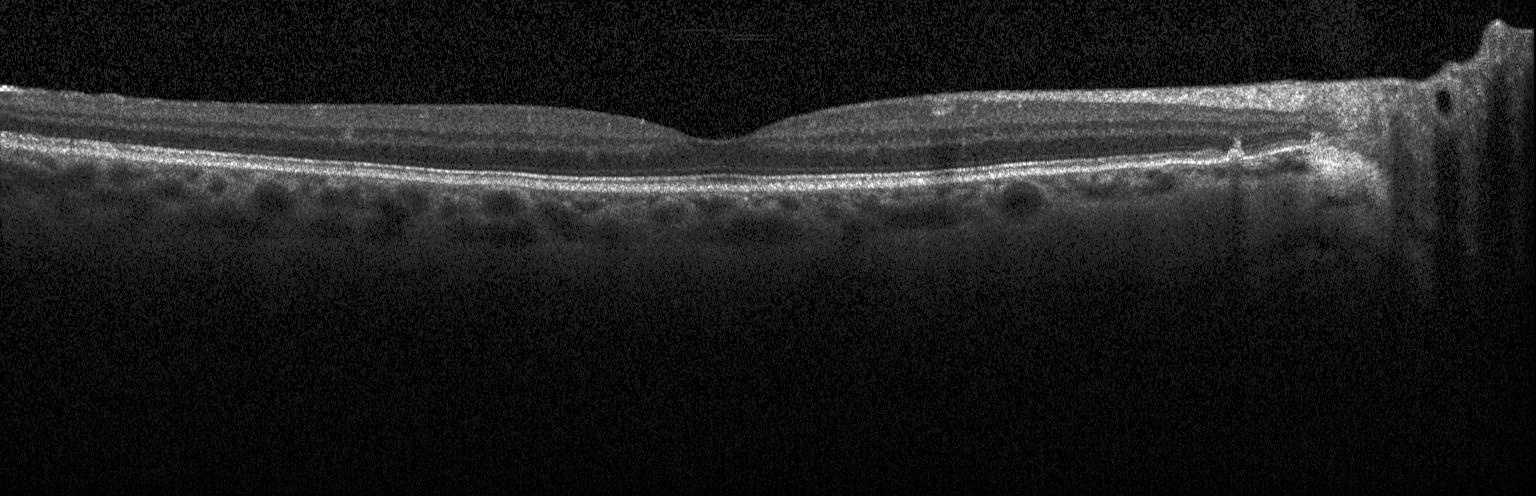 Through the macula; retinal OCT B-scan
This B-scan demonstrates no choroidal neovascularization, no diabetic macular edema, and no drusen.